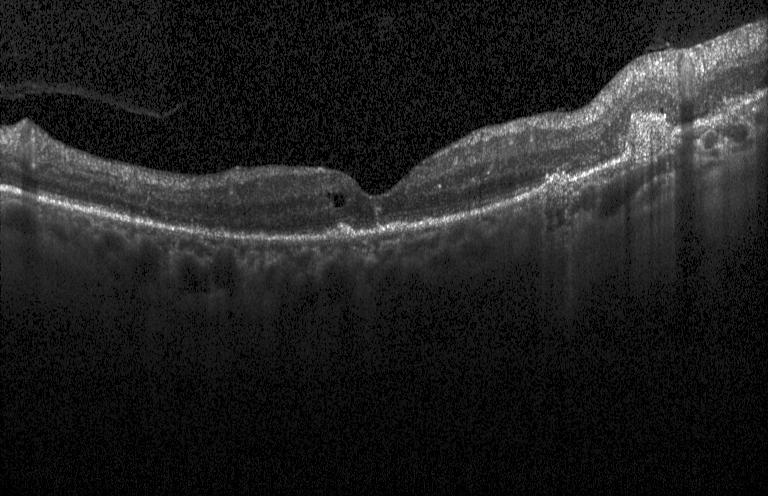
OCT line scan. Dx: choroidal neovascularization.